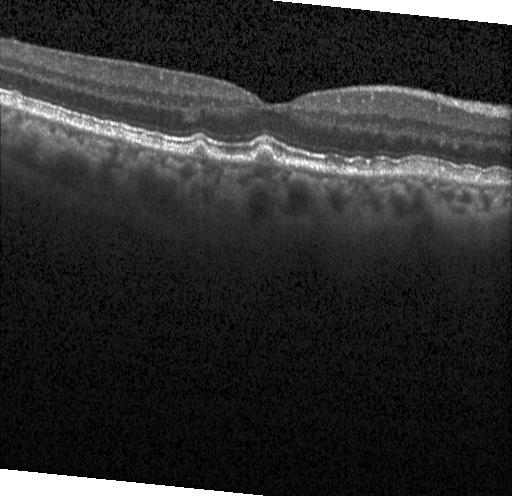

Optical coherence tomography scan.
Impression: multiple drusen.